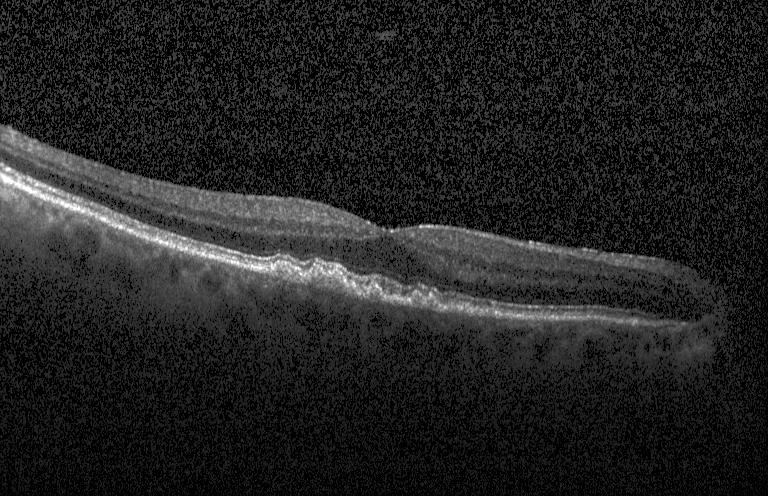
Diagnosis: multiple drusen.